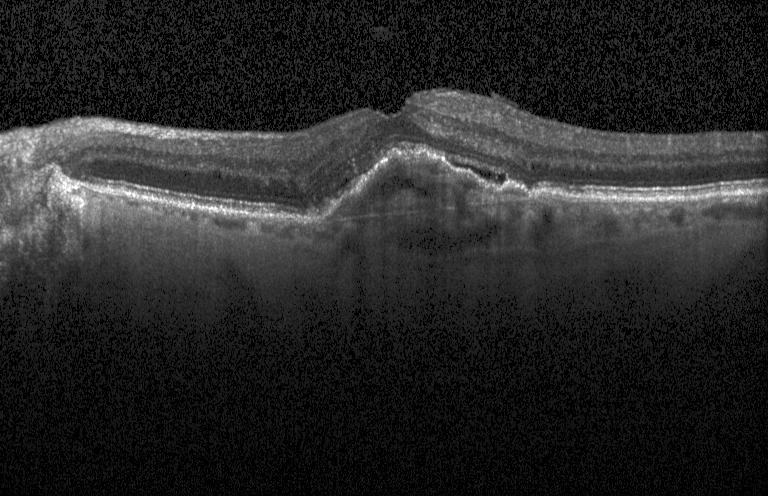
OCT B-scan showing a choroidal neovascular membrane.